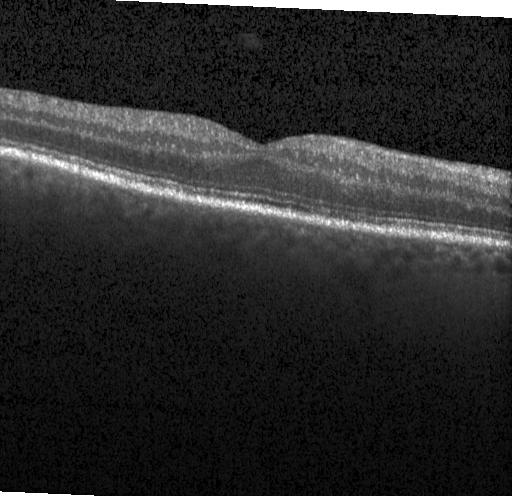
OCT B-scan showing no CNV, DME, or drusen.